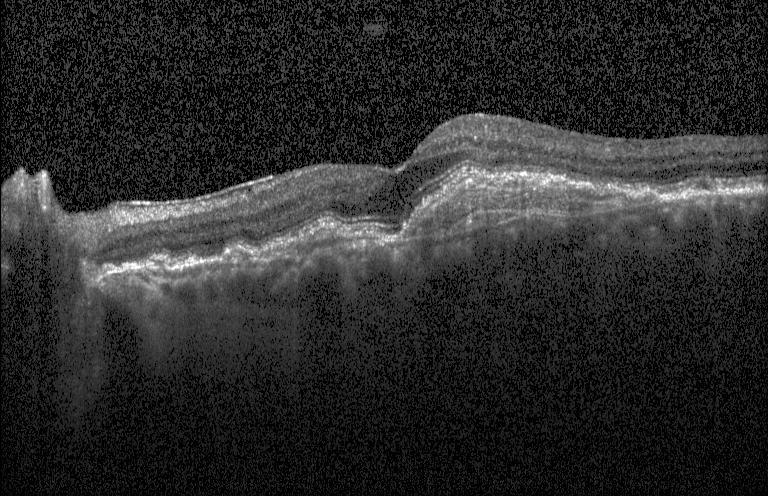
Macular OCT demonstrating a choroidal neovascular membrane.